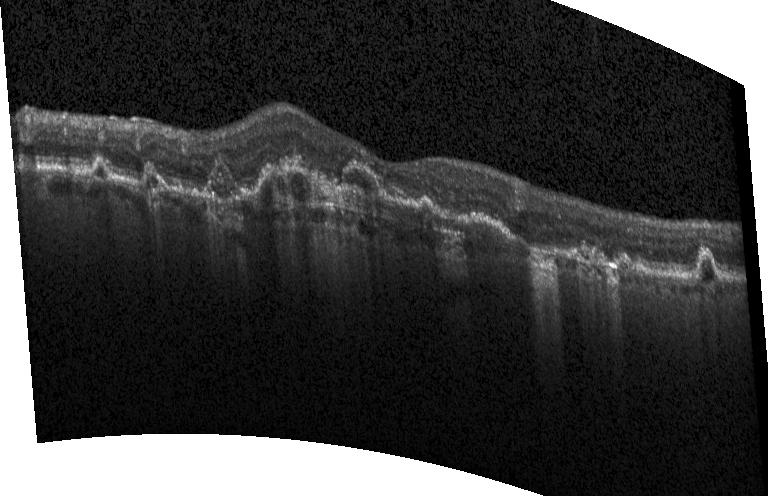 Heidelberg Spectralis; OCT line scan; spectral-domain optical coherence tomography; macular scan. Diagnosis: choroidal neovascularization (CNV).